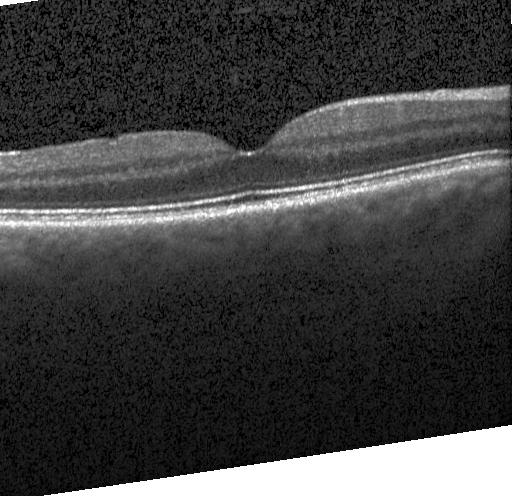

Optical coherence tomography scan.
No CNV, DME, or drusen.